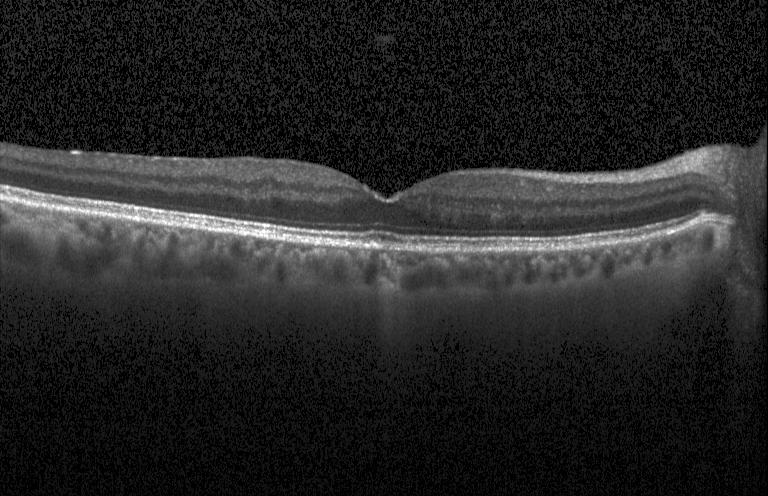
Optical coherence tomography B-scan, horizontal scan through the fovea, SD-OCT
OCT finding: no CNV, DME, or drusen.